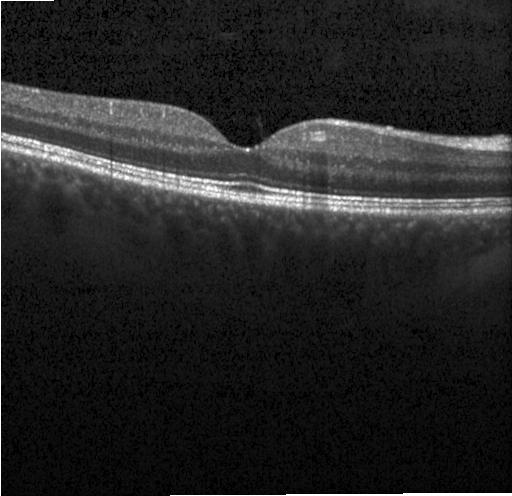

Impression: no choroidal neovascularization, no diabetic macular edema, and no drusen.